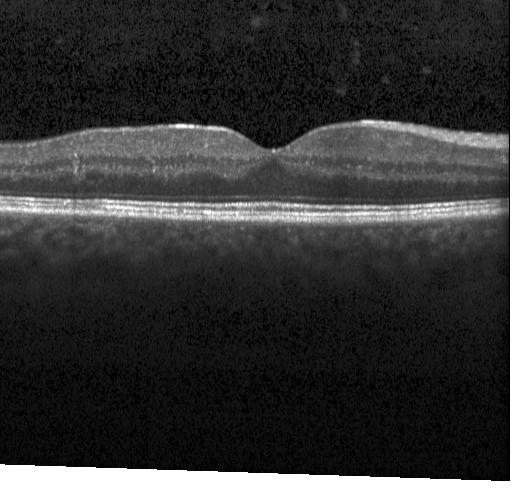 Instrument: Heidelberg Spectralis · retinal OCT B-scan
Assessment: no evidence of CNV, DME, or drusen.